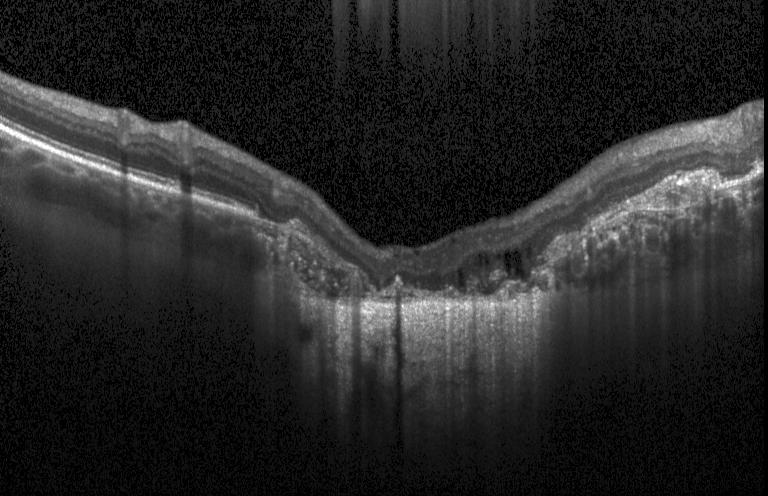
Instrument: Heidelberg Spectralis, SD-OCT, fovea-centered, optical coherence tomography scan.
Diagnosis: choroidal neovascularization.